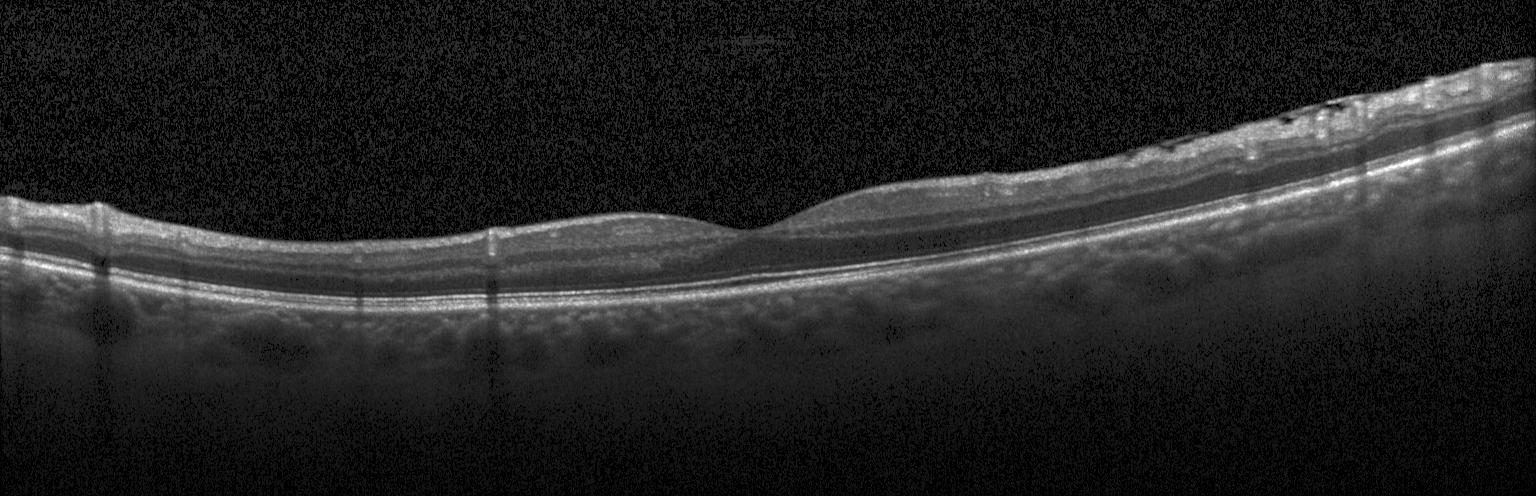
Macular OCT demonstrating neither choroidal neovascularization, diabetic macular edema, nor drusen.